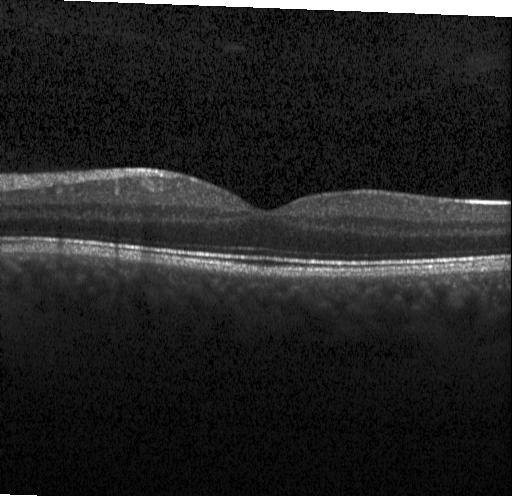 Instrument: Heidelberg Spectralis. Centered on the fovea. OCT line scan. Assessment: no choroidal neovascularization, no diabetic macular edema, and no drusen.